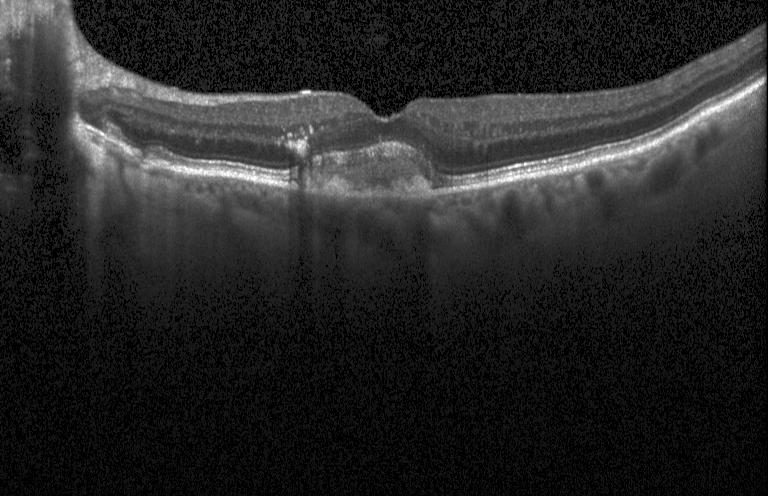
Diagnosis: CNV.